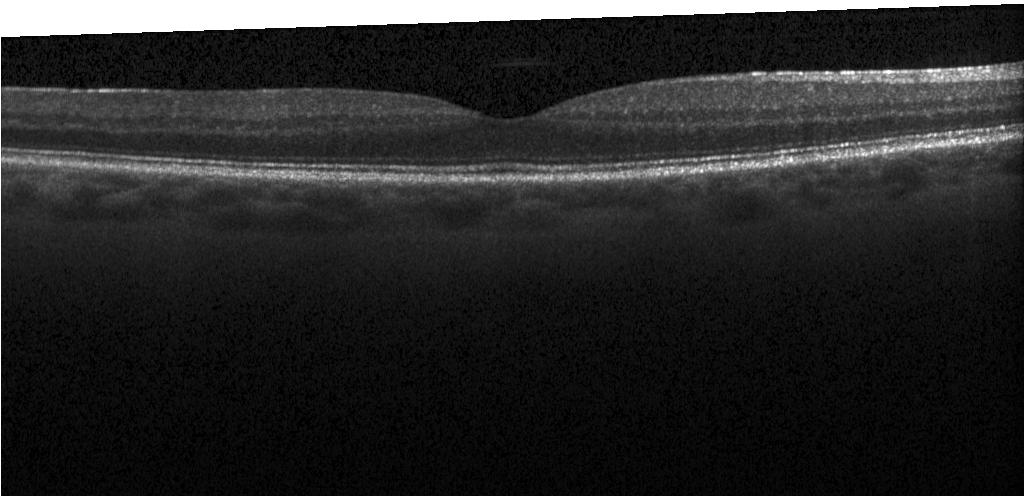
OCT finding: no choroidal neovascularization, diabetic macular edema, or drusen.